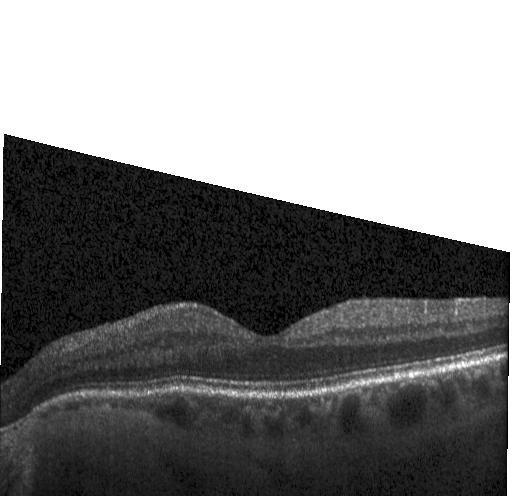

The scan shows no choroidal neovascularization, diabetic macular edema, or drusen.